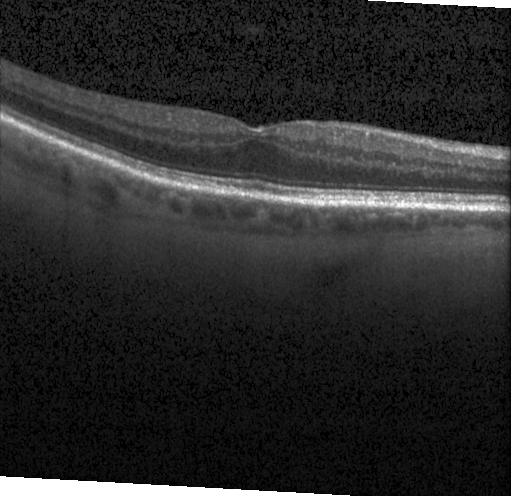 Macular scan. Heidelberg Spectralis. OCT line scan. SD-OCT. No CNV, no DME, and no drusen.